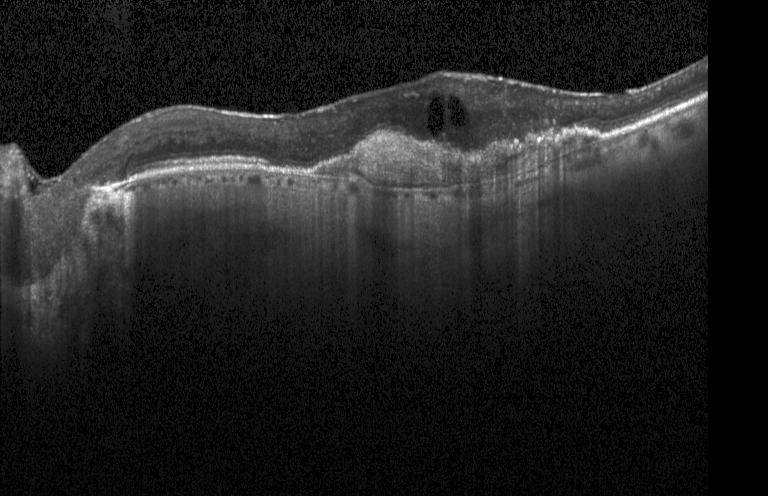
OCT B-scan showing a choroidal neovascular membrane.